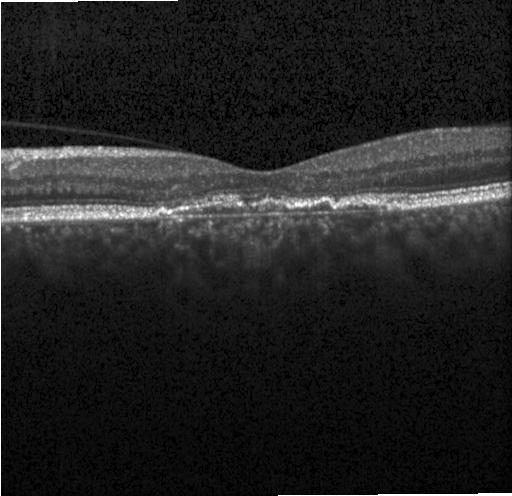
Instrument: Heidelberg Spectralis, optical coherence tomography scan.
The scan shows choroidal neovascularization (CNV).